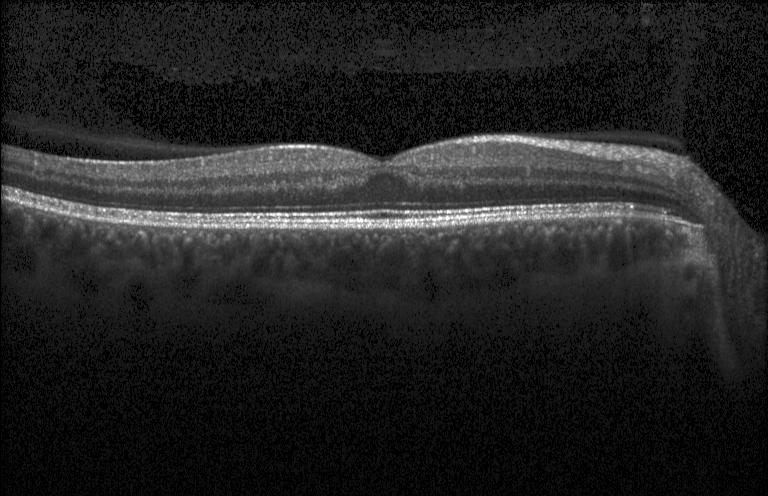
Optical coherence tomography scan; SD-OCT; Heidelberg Spectralis; macular scan — Diagnosis: no evidence of choroidal neovascularization, diabetic macular edema, or drusen.